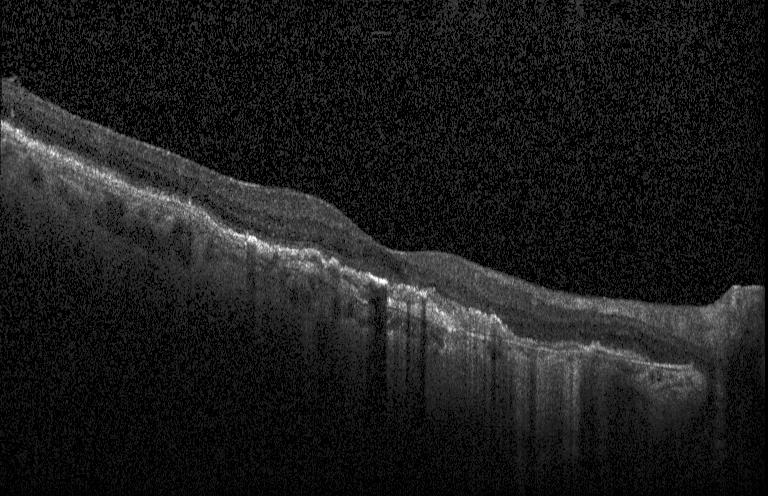
Macular scan · retinal OCT cross-section · SD-OCT — This B-scan demonstrates a choroidal neovascular membrane.